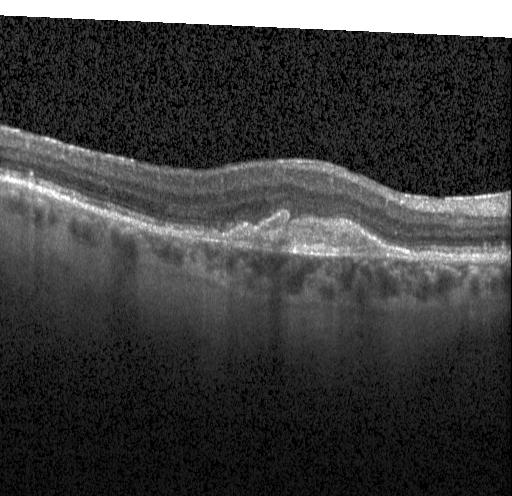 Spectral-domain optical coherence tomography. Macular scan. Retinal OCT cross-section. Instrument: Heidelberg Spectralis
The scan shows a choroidal neovascular membrane.